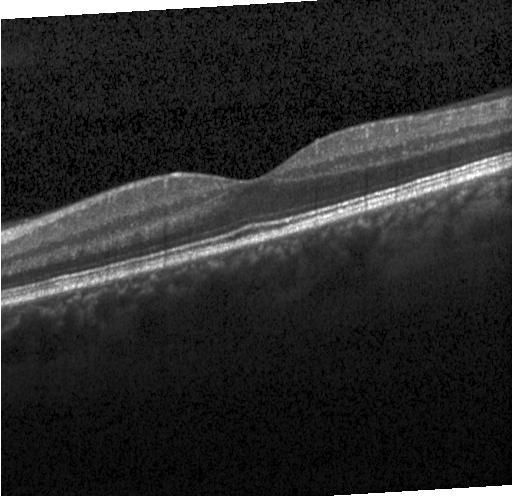
Horizontal scan through the fovea; retinal OCT cross-section. Finding: neither choroidal neovascularization, diabetic macular edema, nor drusen.